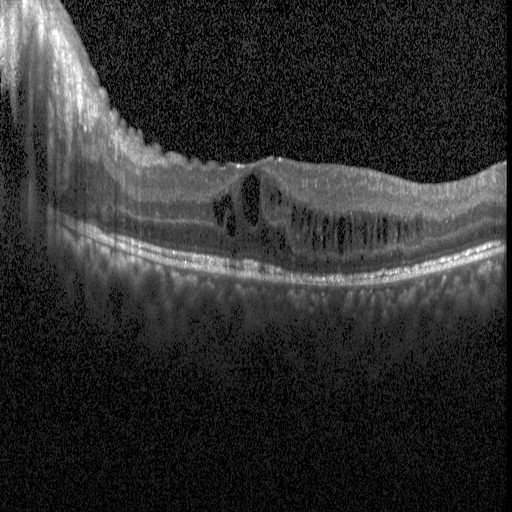 Optical coherence tomography scan. Centered on the fovea. Impression: diabetic macular edema.